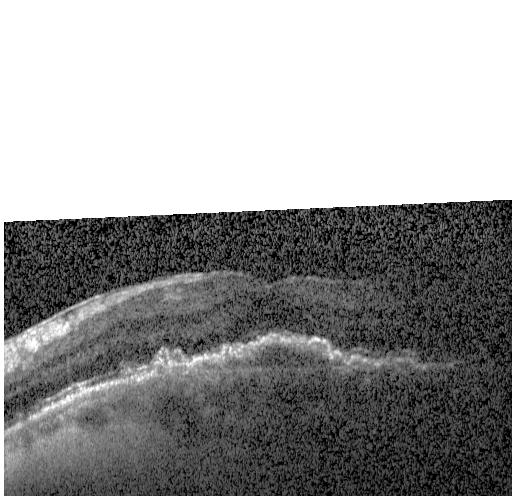 Spectral-domain OCT · Heidelberg Spectralis OCT system · horizontal scan through the fovea · OCT B-scan.
Impression: choroidal neovascularization (CNV).